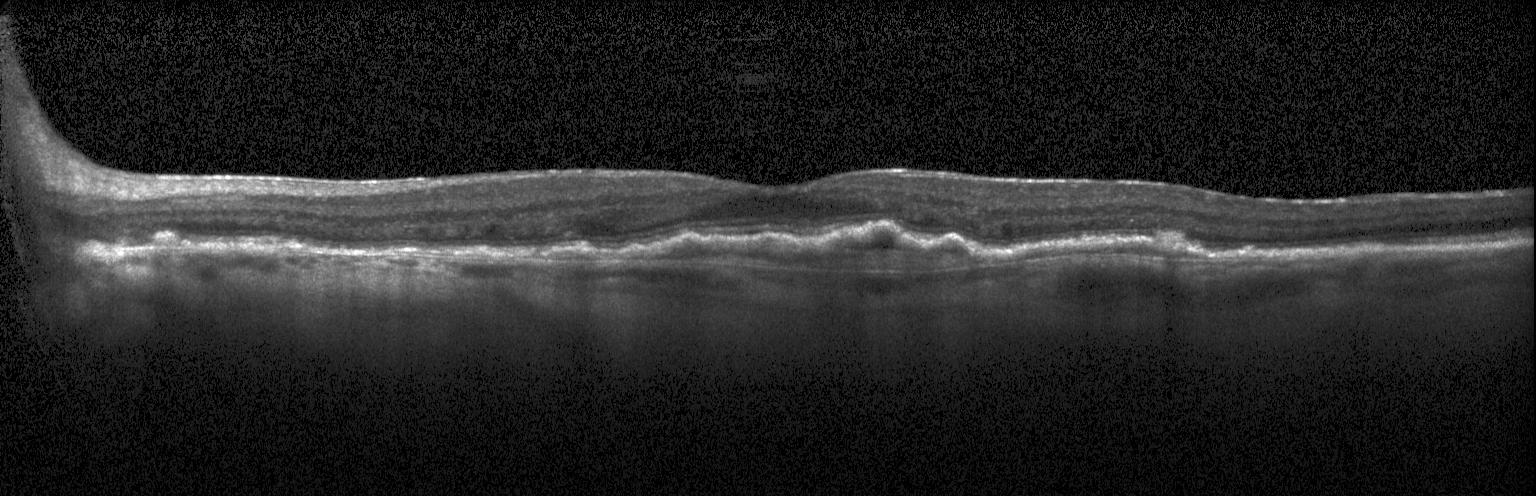
Macular scan; optical coherence tomography scan
Diagnosis: a choroidal neovascular membrane.